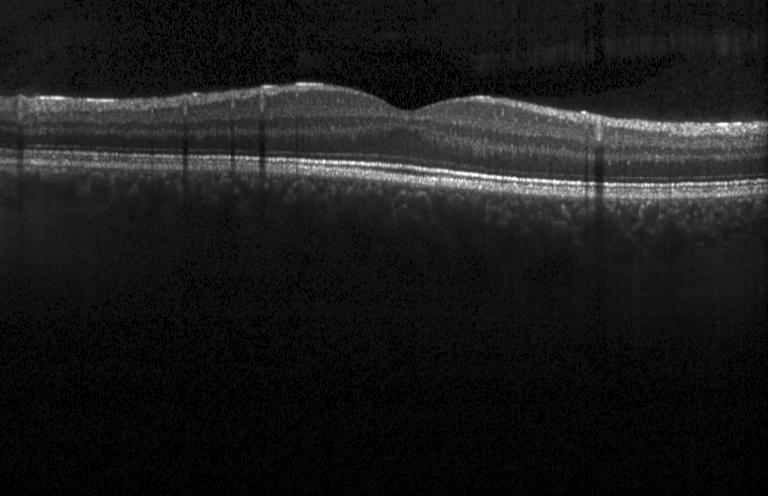
Optical coherence tomography scan; SD-OCT.
The scan shows no CNV, no DME, and no drusen.